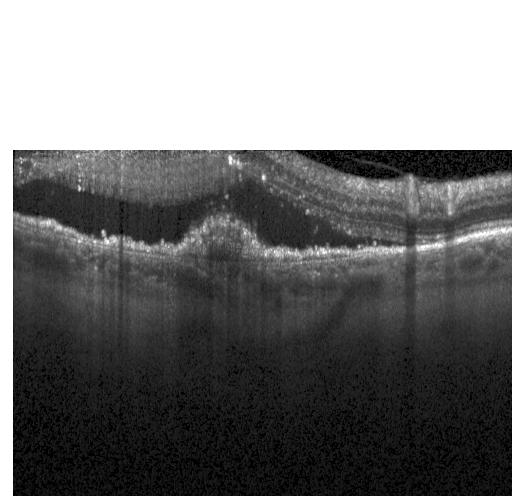 Macular scan · OCT line scan.
Diagnosis: choroidal neovascularization.